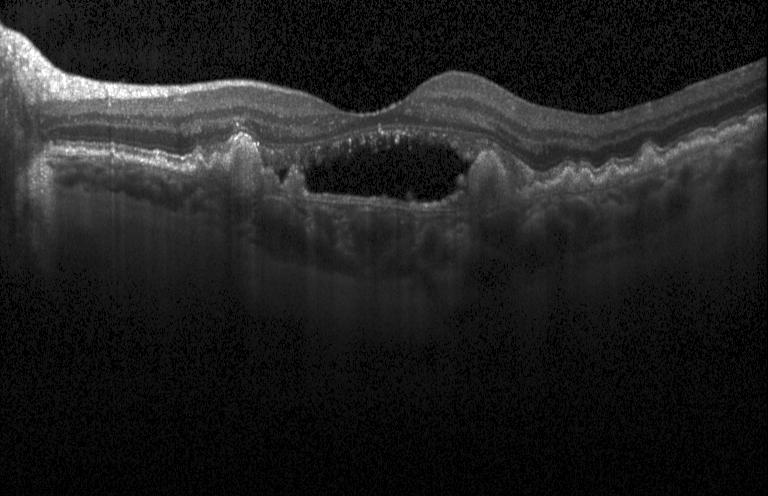
Impression: CNV.